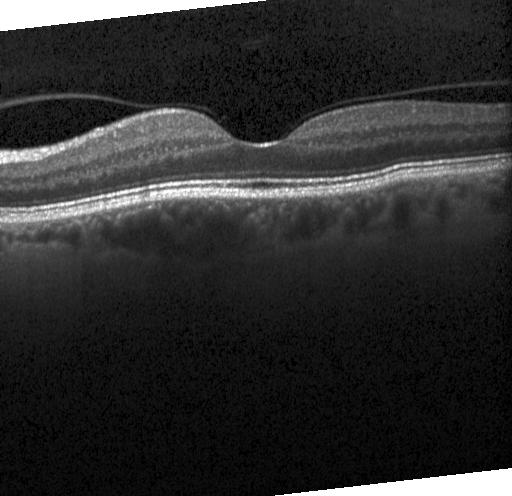
Macular OCT: no CNV, DME, or drusen.